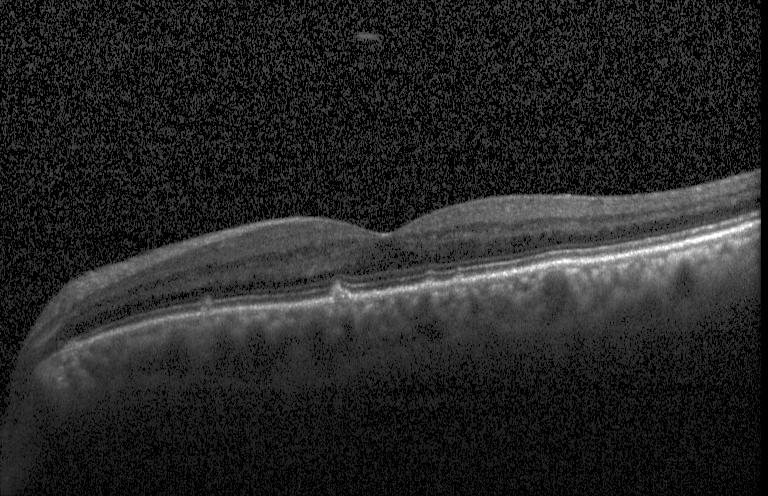

Centered on the fovea; retinal OCT B-scan. Finding: drusen.